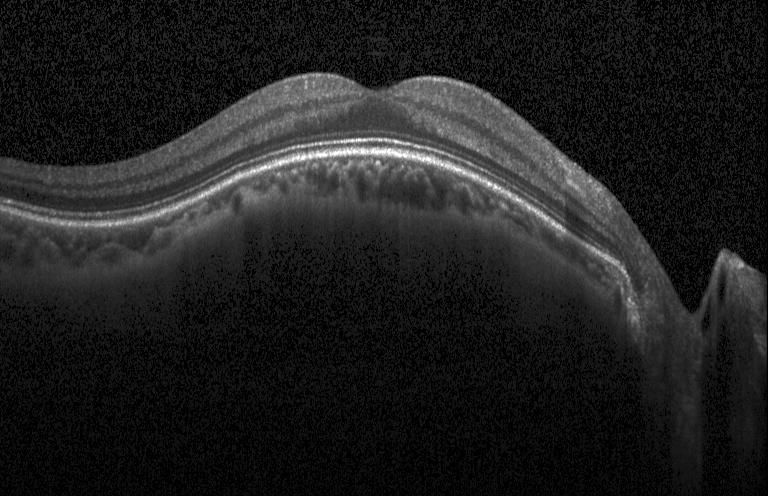 Diagnosis: no evidence of choroidal neovascularization, diabetic macular edema, or drusen.